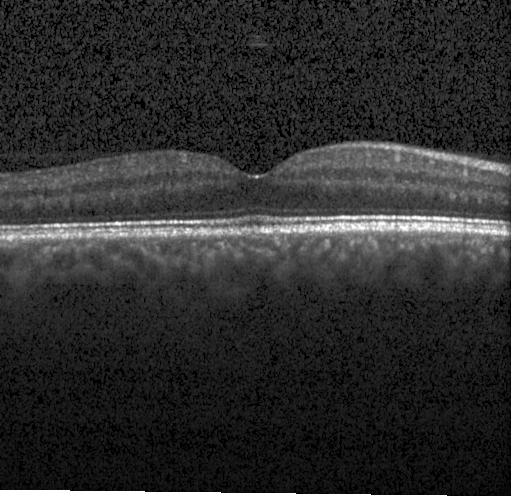 Optical coherence tomography B-scan · macular scan. Macular OCT: no CNV, no DME, and no drusen.